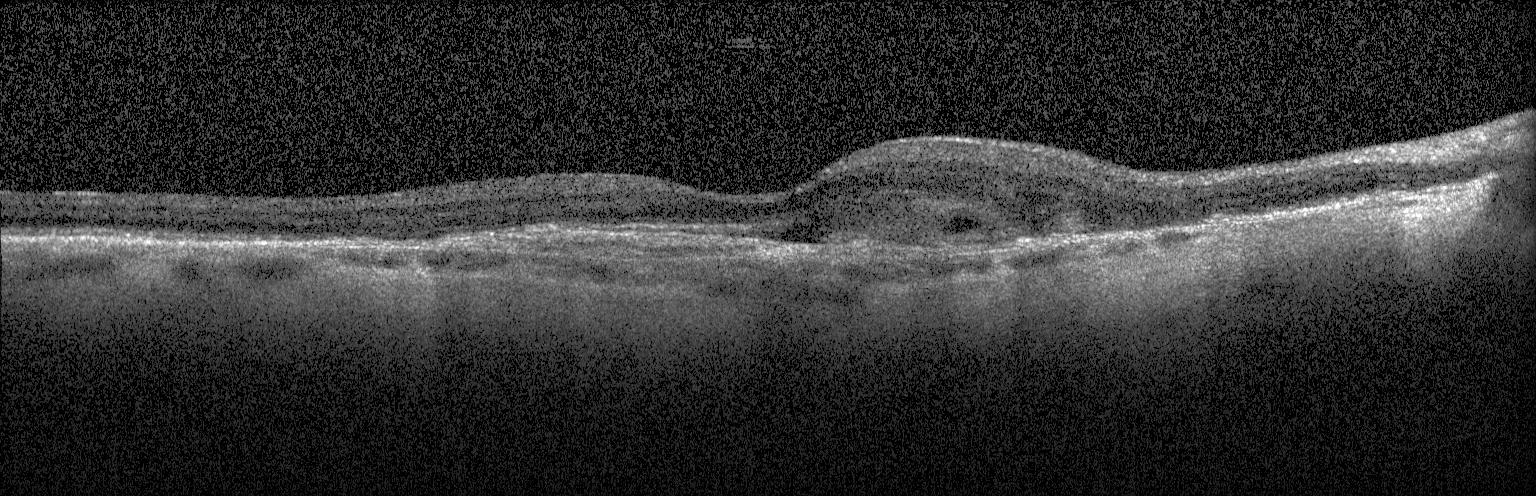 Retinal OCT cross-section showing a choroidal neovascular membrane.